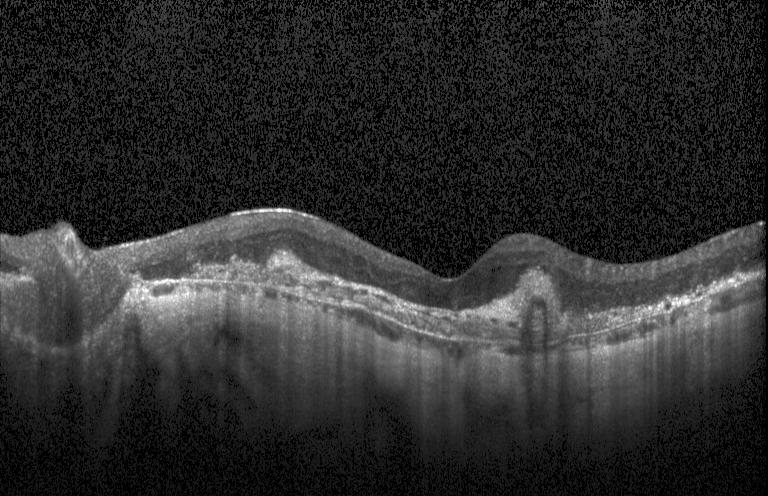 Spectral-domain OCT B-scan: choroidal neovascularization (CNV).